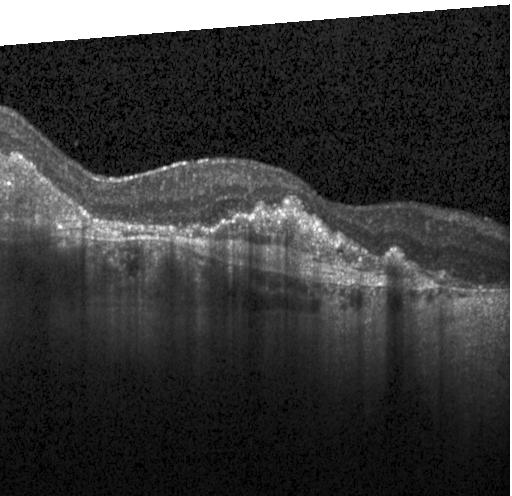
Retinal OCT cross-section showing choroidal neovascularization (CNV).